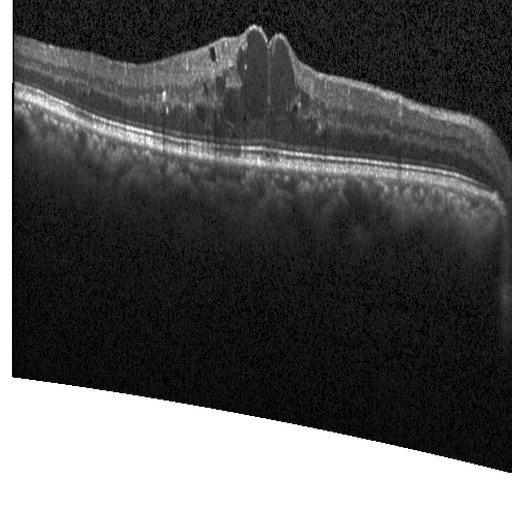
Diagnosis: DME.